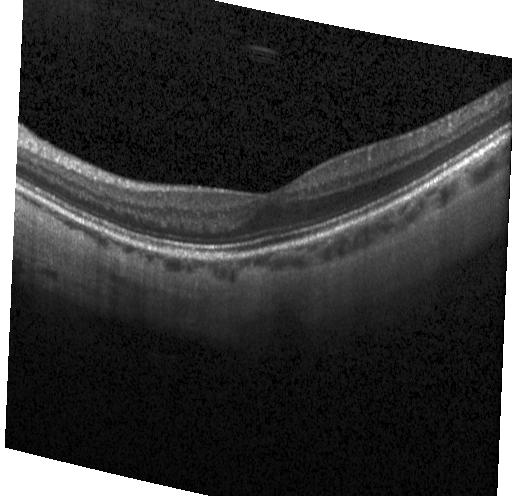
Optical coherence tomography B-scan. Spectral-domain OCT
This B-scan demonstrates no evidence of choroidal neovascularization, diabetic macular edema, or drusen.